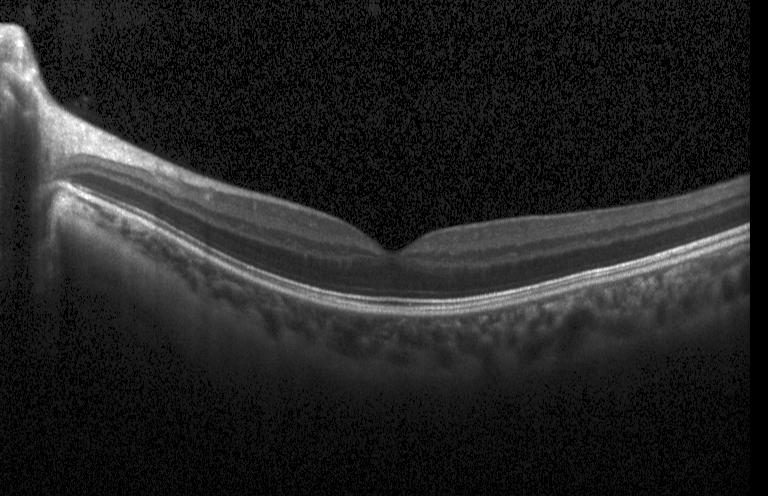
Spectral-domain OCT. Instrument: Heidelberg Spectralis. Fovea-centered. Optical coherence tomography scan.
OCT finding: neither CNV, DME, nor drusen.